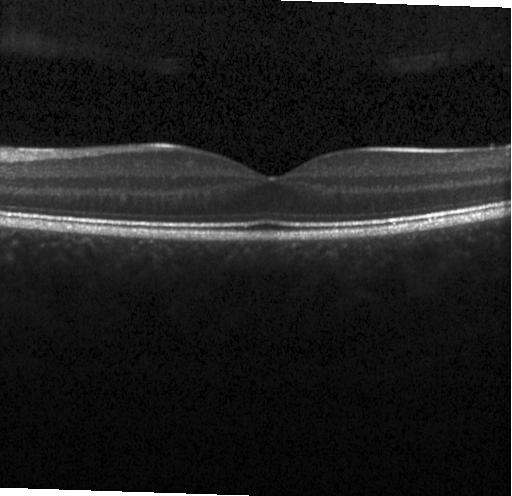
OCT B-scan, spectral-domain optical coherence tomography, fovea-centered
Impression: neither CNV, DME, nor drusen.